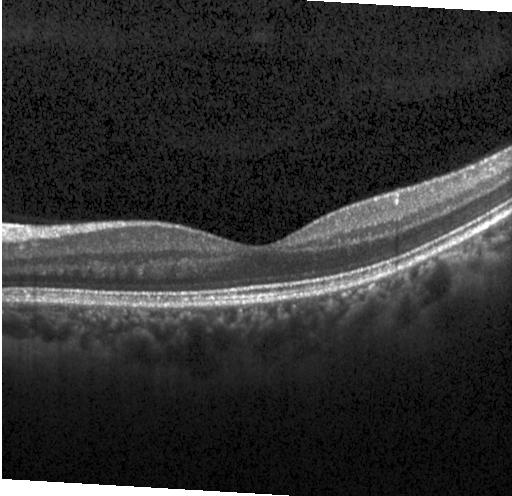
No choroidal neovascularization, no diabetic macular edema, and no drusen.